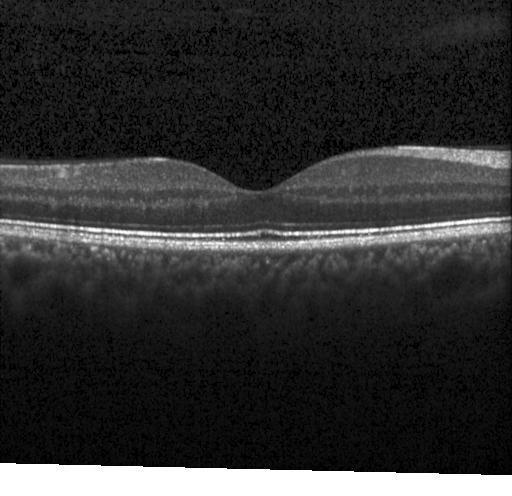
Optical coherence tomography B-scan, spectral-domain optical coherence tomography — The scan shows no CNV, no DME, and no drusen.